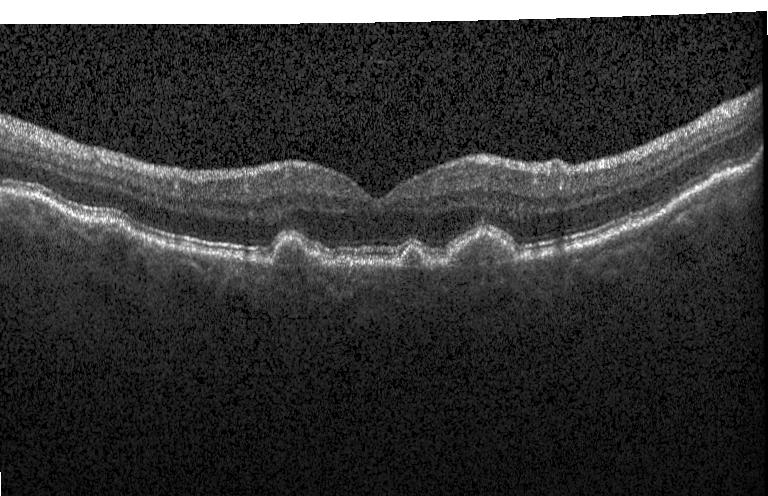

Spectral-domain optical coherence tomography. OCT line scan. Fovea-centered.
Dx: sub-RPE drusenoid deposits.